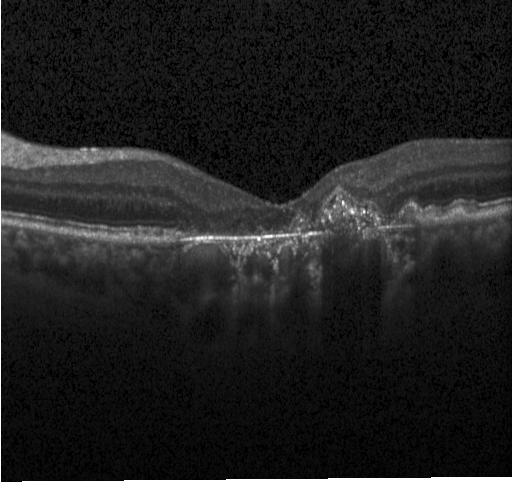 Diagnosis: a choroidal neovascular membrane.